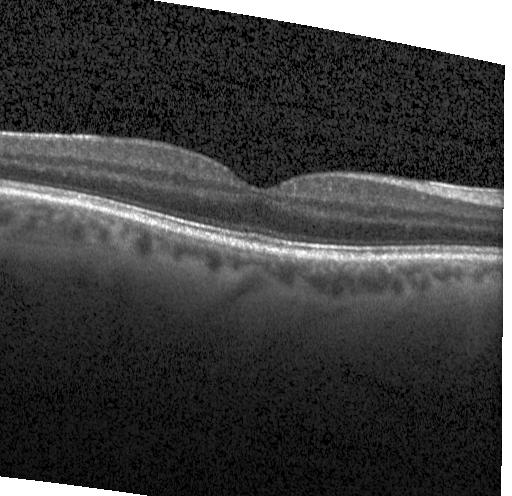
Retinal OCT B-scan.
OCT finding: no CNV, no DME, and no drusen.